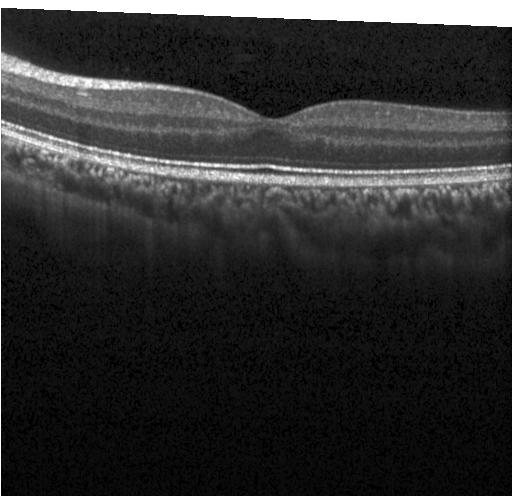 Optical coherence tomography B-scan
Finding: no evidence of choroidal neovascularization, diabetic macular edema, or drusen.